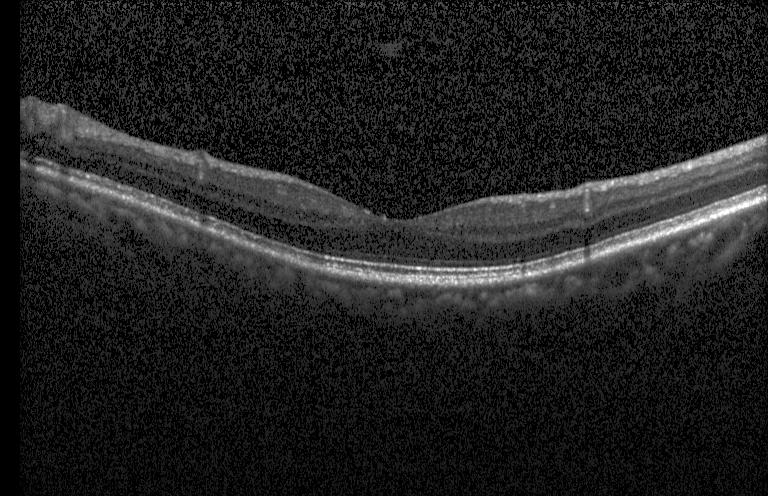
Horizontal scan through the fovea, retinal OCT B-scan, acquired on a Heidelberg Spectralis, spectral-domain optical coherence tomography.
No choroidal neovascularization, diabetic macular edema, or drusen.